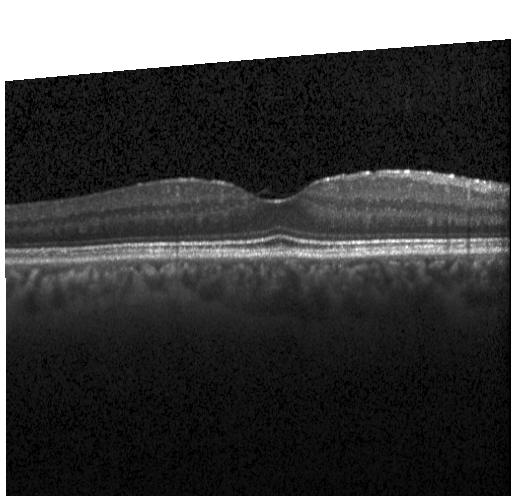

Spectral-domain optical coherence tomography. Retinal OCT cross-section. Heidelberg Spectralis. Macular scan. This B-scan demonstrates no evidence of choroidal neovascularization, diabetic macular edema, or drusen.